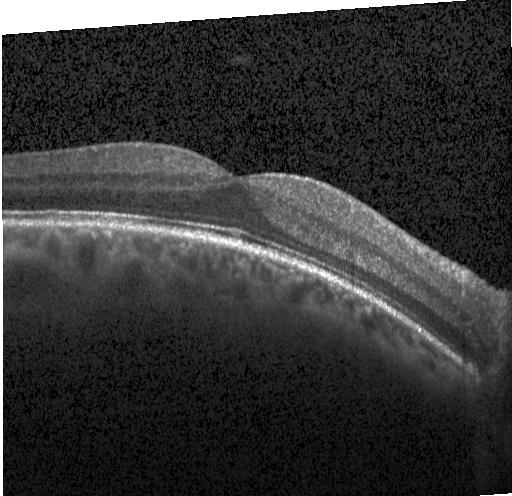 Instrument: Heidelberg Spectralis, retinal OCT cross-section, horizontal scan through the fovea. Impression: no CNV, no DME, and no drusen.